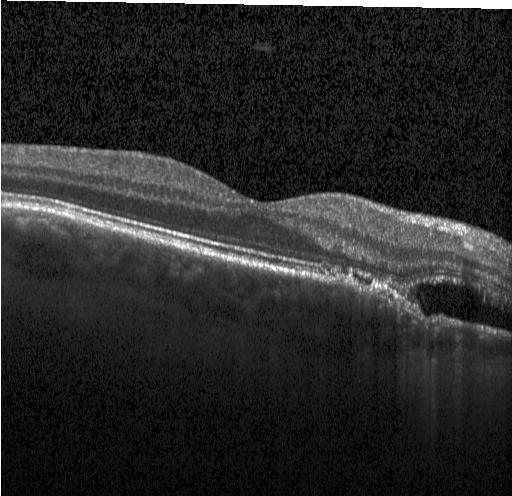
Retinal OCT cross-section · instrument: Heidelberg Spectralis · spectral-domain OCT
Impression: a choroidal neovascular membrane.